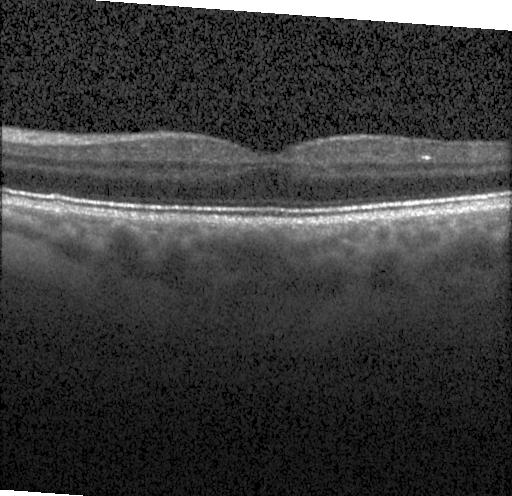
Optical coherence tomography B-scan; Heidelberg Spectralis OCT system; centered on the fovea. Impression: no evidence of choroidal neovascularization, diabetic macular edema, or drusen.